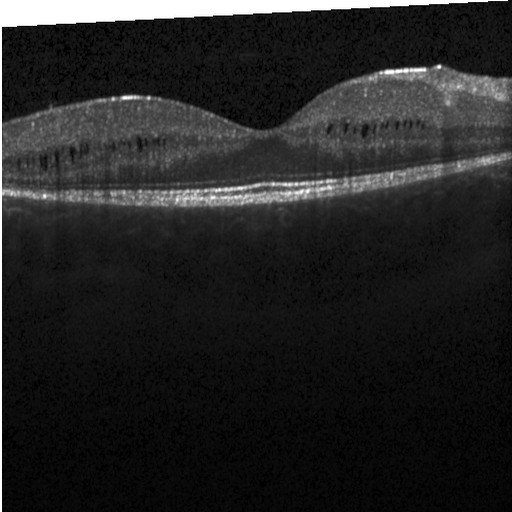 Impression: DME.